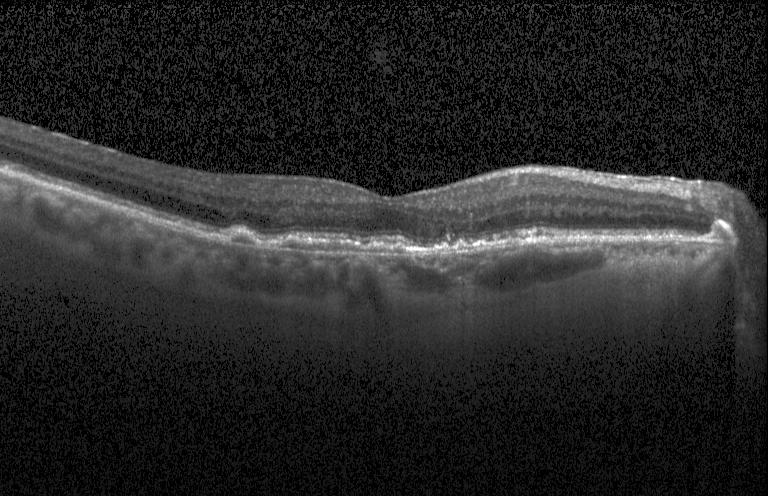 OCT line scan. Spectral-domain optical coherence tomography — Finding: choroidal neovascularization (CNV).